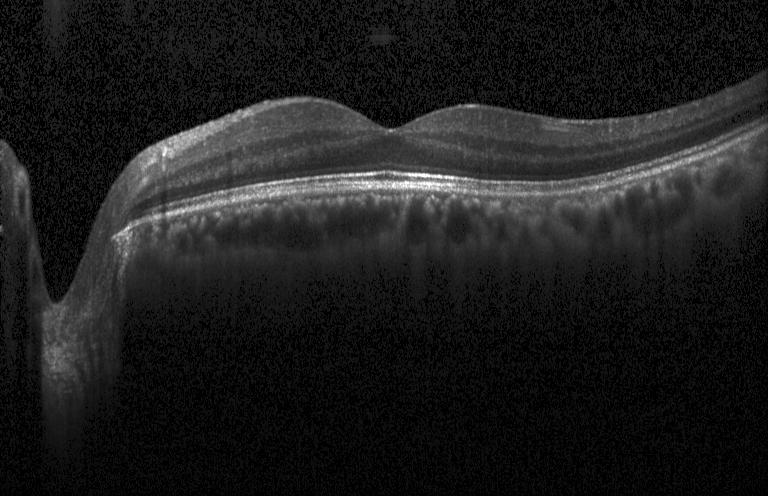 Spectral-domain OCT · through the macula · Heidelberg Spectralis OCT system · optical coherence tomography scan
This B-scan demonstrates no CNV, no DME, and no drusen.